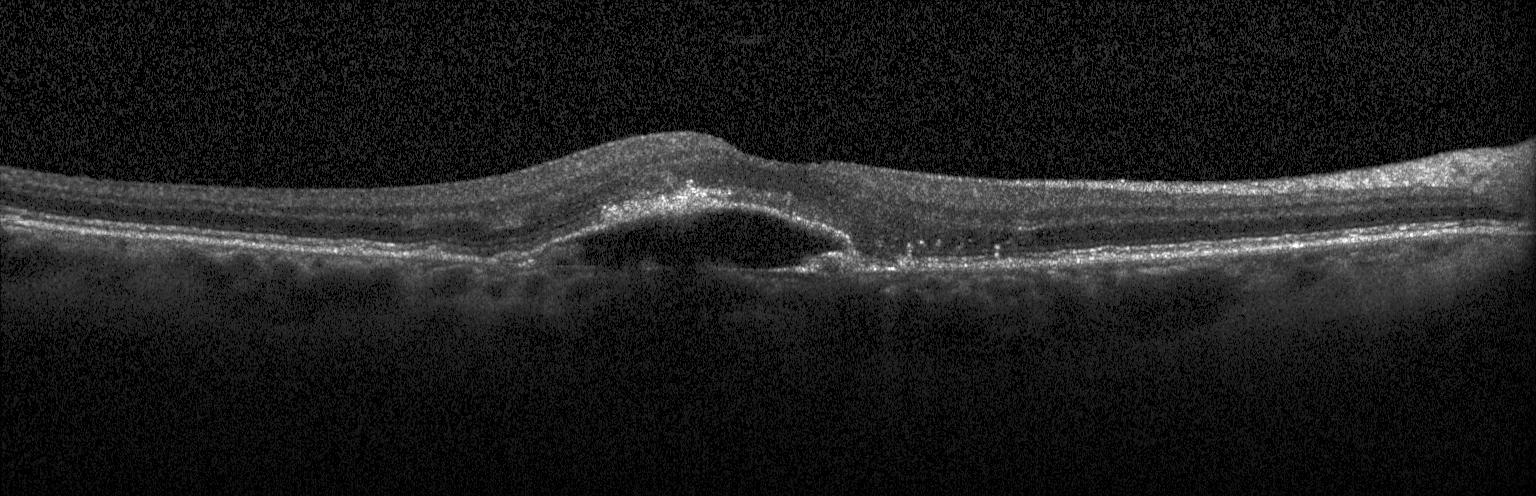

OCT line scan, acquired on a Heidelberg Spectralis. Assessment: a choroidal neovascular membrane.